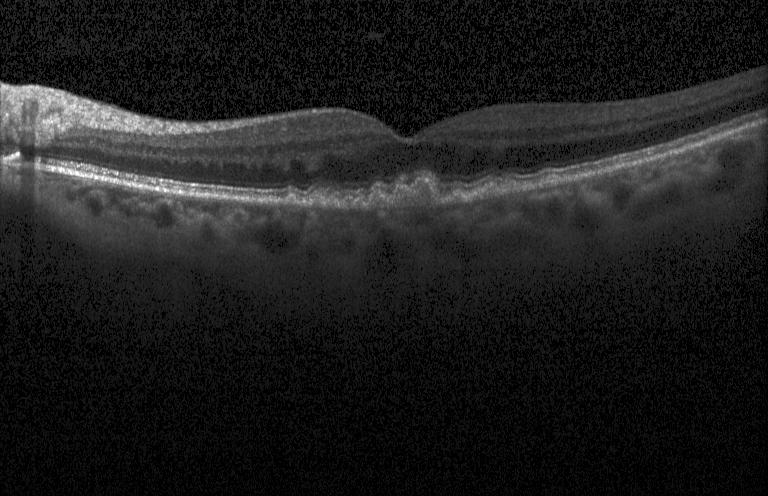
Acquired on a Heidelberg Spectralis; centered on the fovea; SD-OCT; retinal OCT cross-section
Impression: multiple drusen.